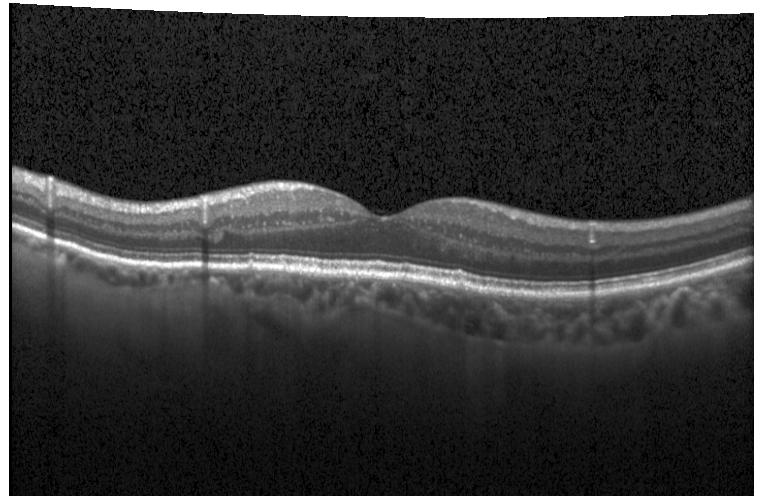
Spectral-domain OCT; macular scan; acquired on a Heidelberg Spectralis; optical coherence tomography B-scan.
Macular OCT: neither CNV, DME, nor drusen.